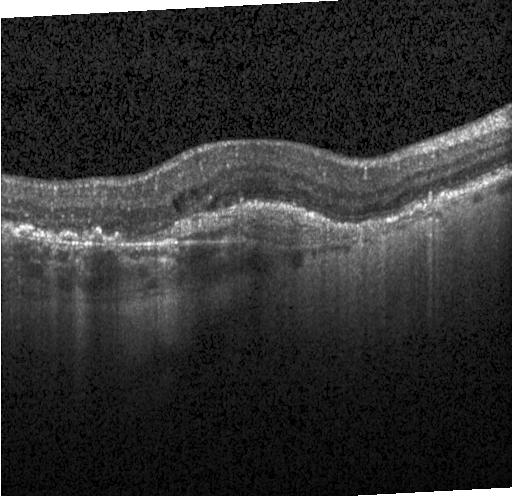
Spectral-domain optical coherence tomography · retinal OCT cross-section.
This B-scan demonstrates CNV.